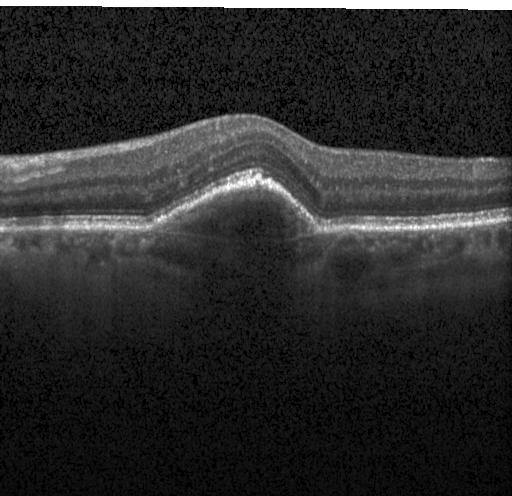

Retinal OCT B-scan
The scan shows a choroidal neovascular membrane.